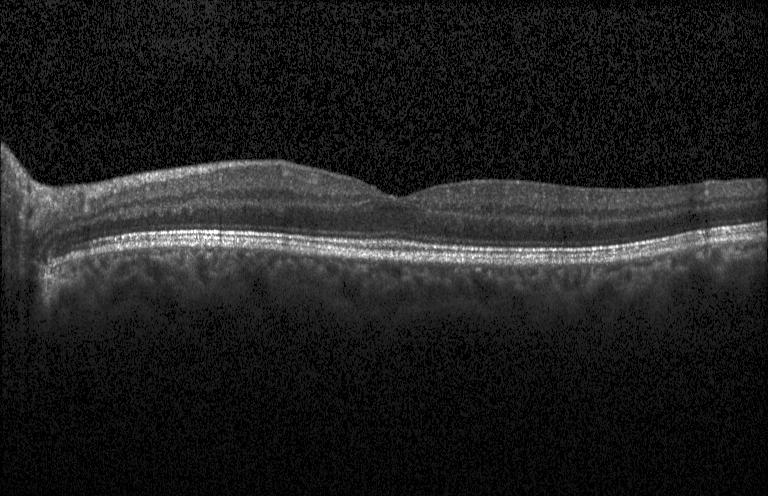

Macular OCT demonstrating no choroidal neovascularization, diabetic macular edema, or drusen.